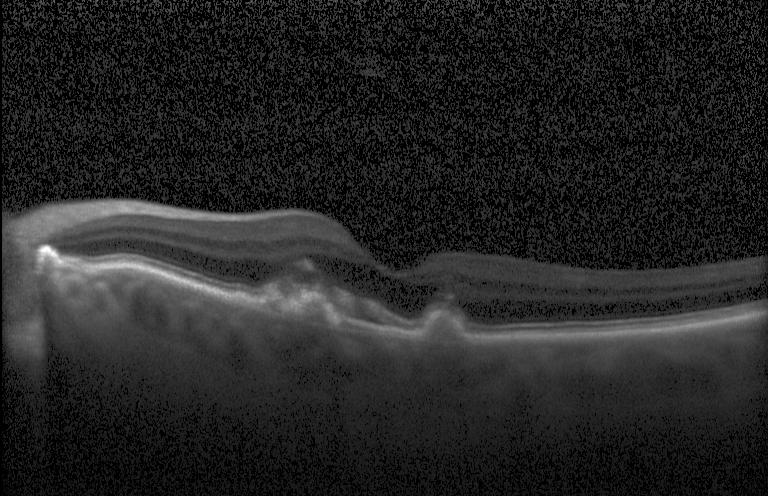

OCT B-scan showing CNV.